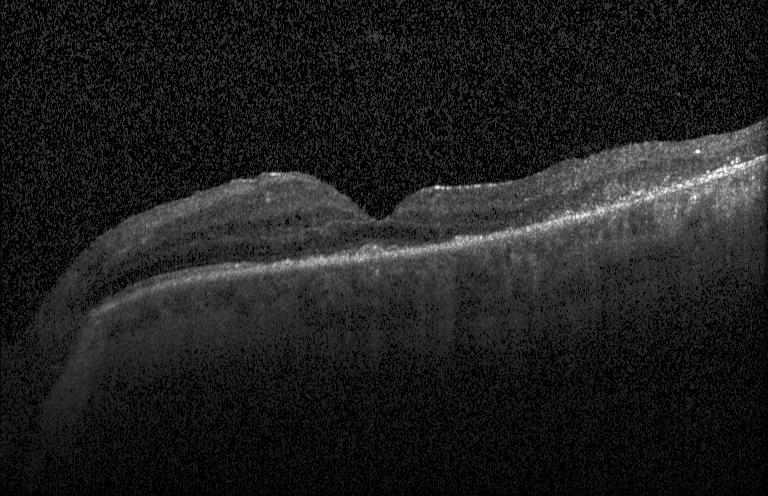

Optical coherence tomography B-scan
Diabetic macular edema.